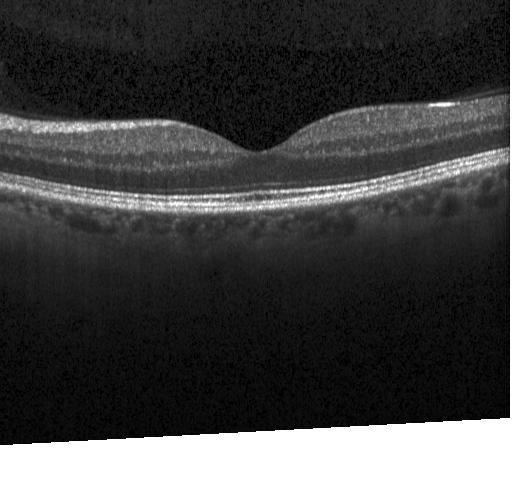

Retinal OCT B-scan. Finding: no choroidal neovascularization, diabetic macular edema, or drusen.